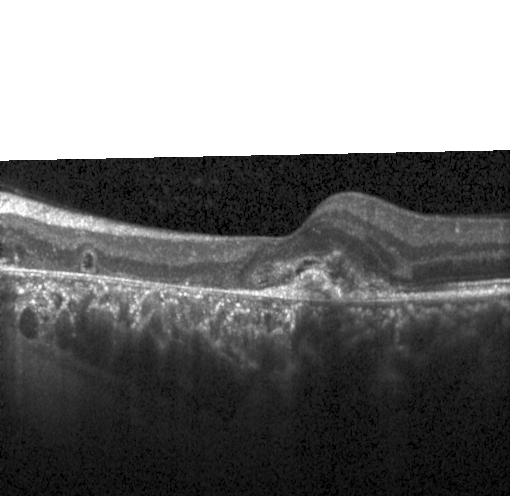 Optical coherence tomography scan; fovea-centered. Finding: a choroidal neovascular membrane.